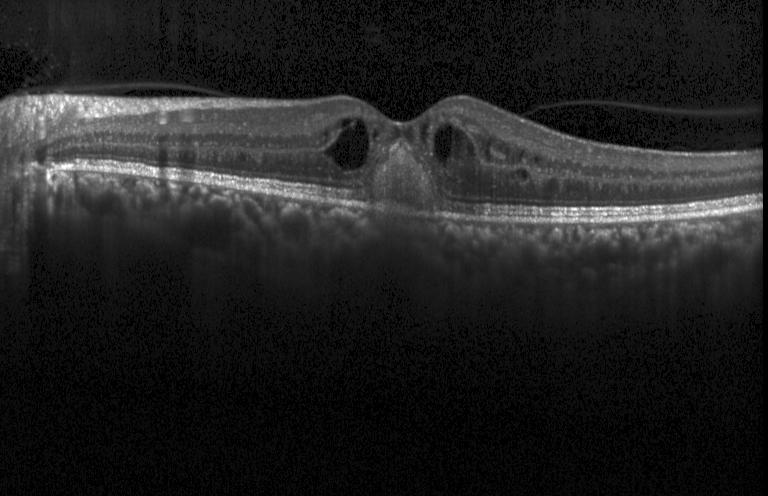
Through the macula, optical coherence tomography B-scan, instrument: Heidelberg Spectralis, SD-OCT.
Assessment: CNV.